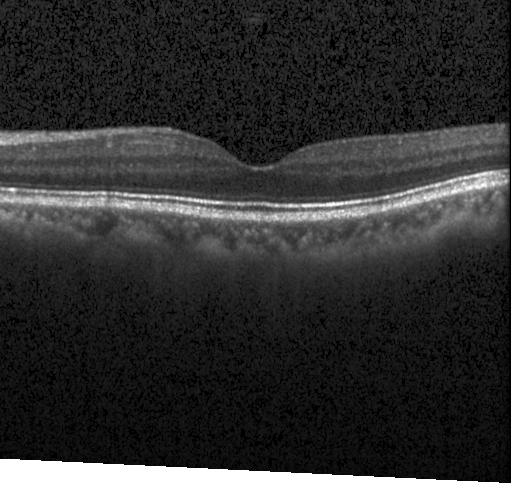
OCT line scan, horizontal scan through the fovea, SD-OCT, Heidelberg Spectralis OCT system. OCT finding: no evidence of choroidal neovascularization, diabetic macular edema, or drusen.